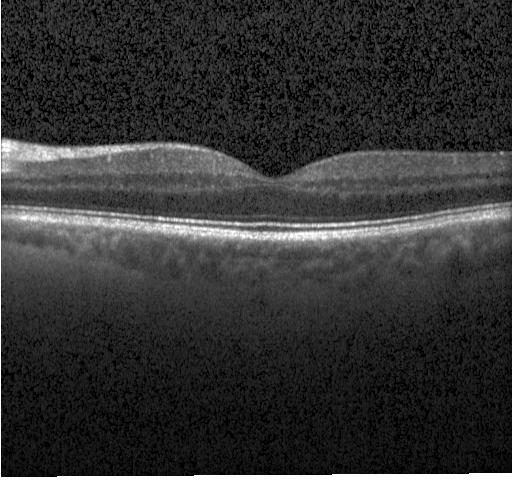

Dx: no choroidal neovascularization, no diabetic macular edema, and no drusen.